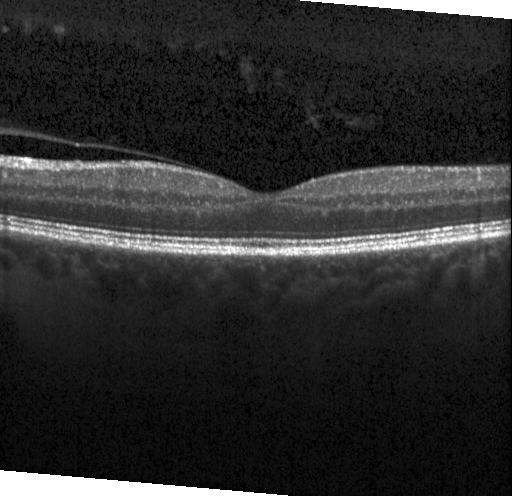
OCT scan showing no evidence of choroidal neovascularization, diabetic macular edema, or drusen.